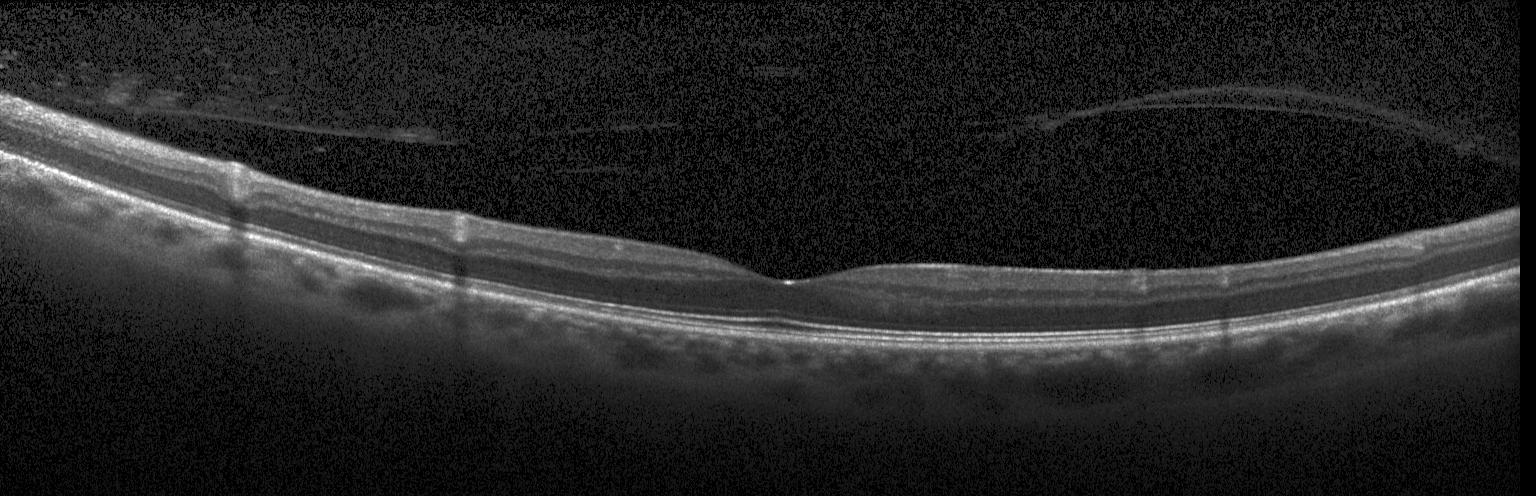
Instrument: Heidelberg Spectralis, fovea-centered, optical coherence tomography B-scan, SD-OCT. Diagnosis: no choroidal neovascularization, diabetic macular edema, or drusen.